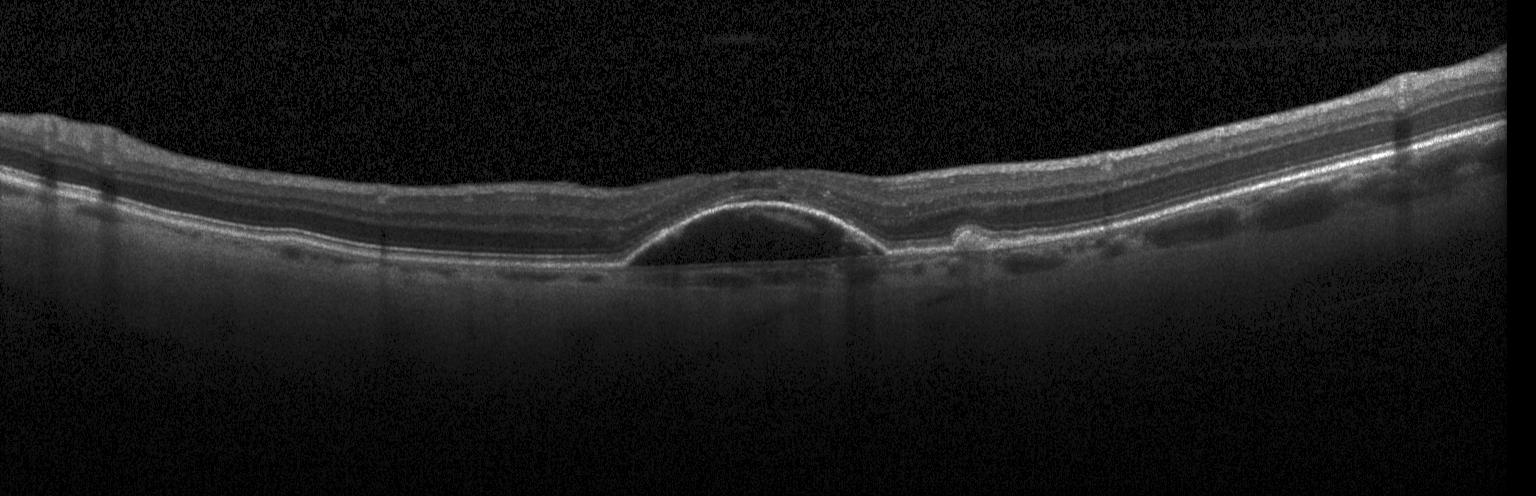 Diagnosis: choroidal neovascularization (CNV).